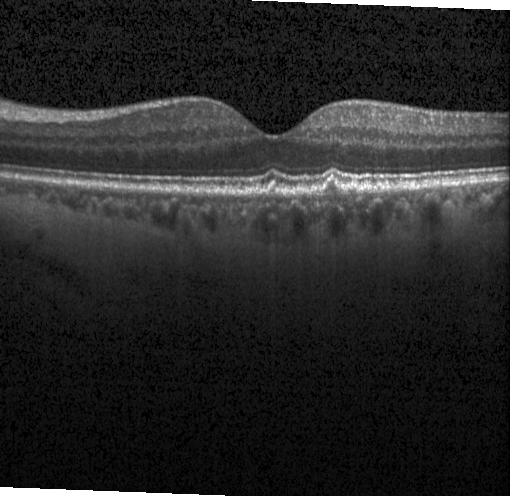 Retinal OCT cross-section.
Diagnosis: drusen.